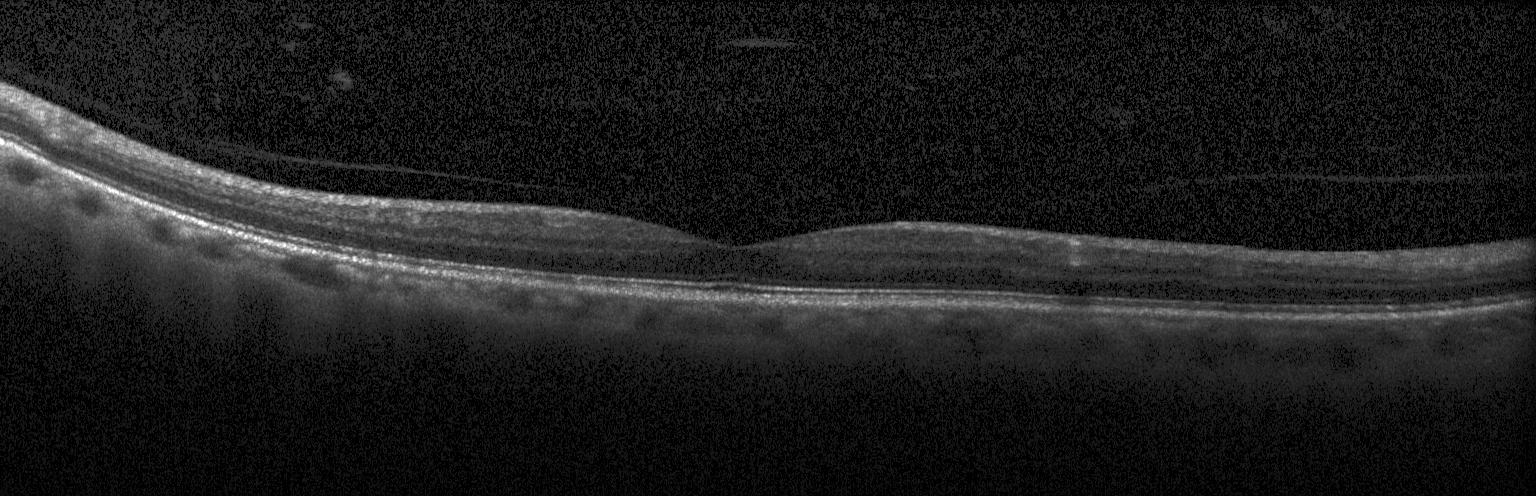

Impression: no choroidal neovascularization, no diabetic macular edema, and no drusen.